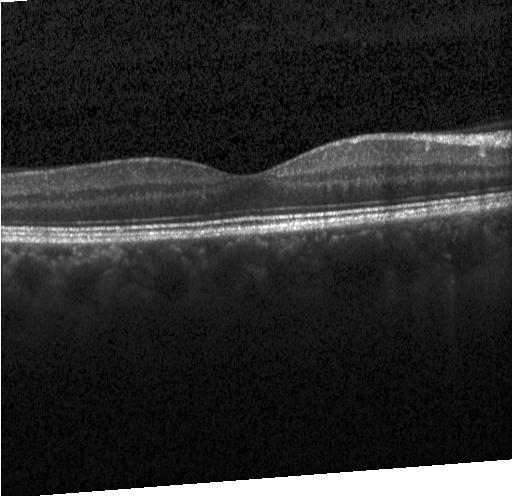 Optical coherence tomography scan
Finding: no choroidal neovascularization, no diabetic macular edema, and no drusen.